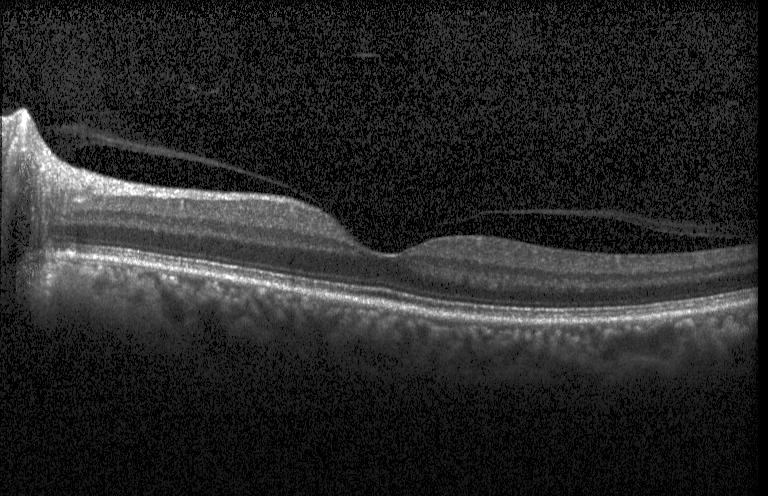 Diagnosis: neither choroidal neovascularization, diabetic macular edema, nor drusen.